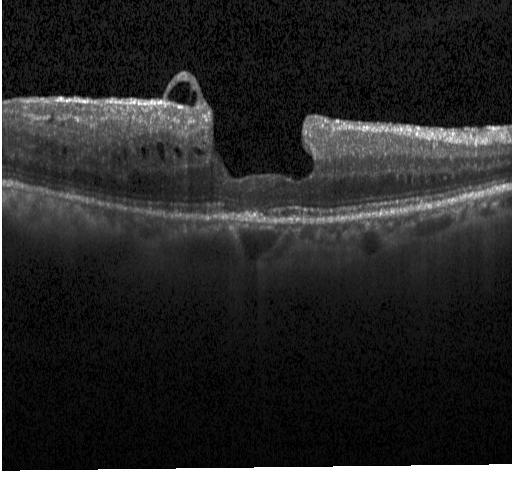

Optical coherence tomography B-scan. Fovea-centered. Spectral-domain optical coherence tomography
Diabetic macular edema.